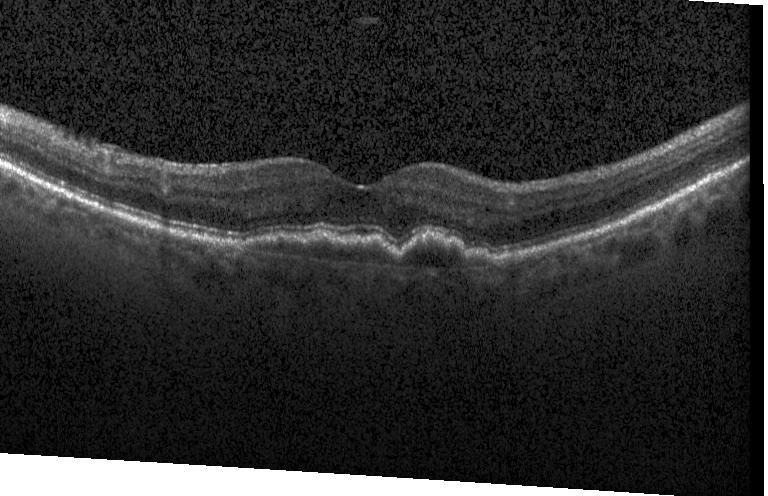
OCT scan showing CNV.